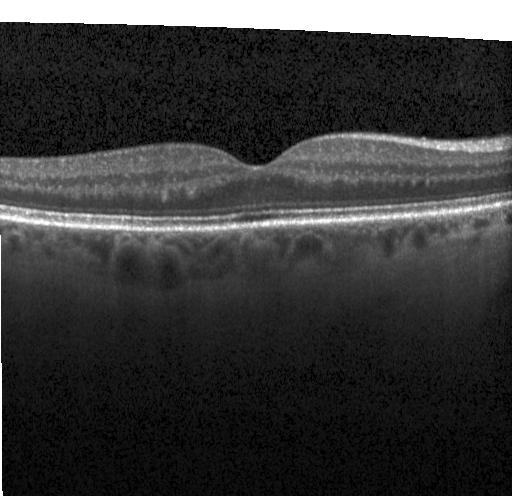
Spectral-domain OCT · optical coherence tomography B-scan · fovea-centered — The scan shows neither CNV, DME, nor drusen.